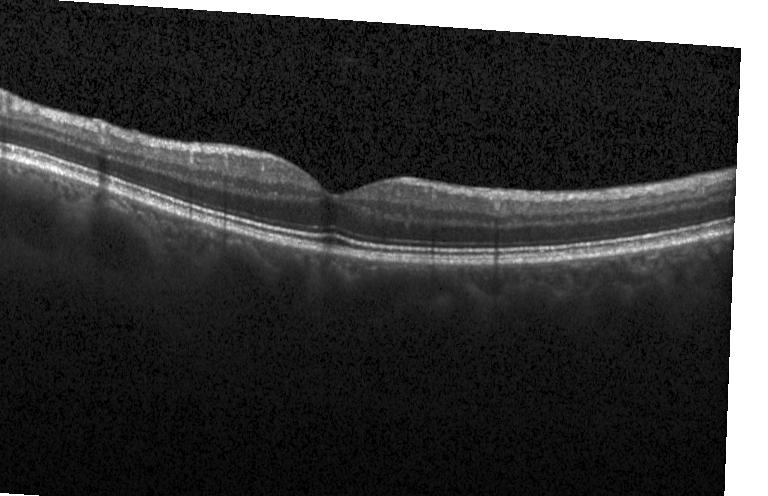
OCT B-scan showing no choroidal neovascularization, no diabetic macular edema, and no drusen.